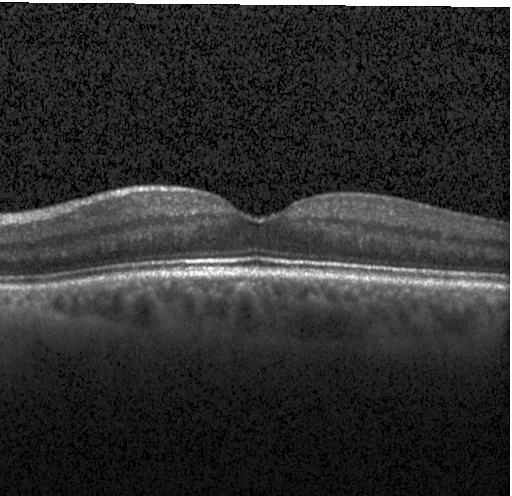
Macular scan, retinal OCT B-scan, Heidelberg Spectralis OCT system, spectral-domain optical coherence tomography — Finding: no evidence of choroidal neovascularization, diabetic macular edema, or drusen.